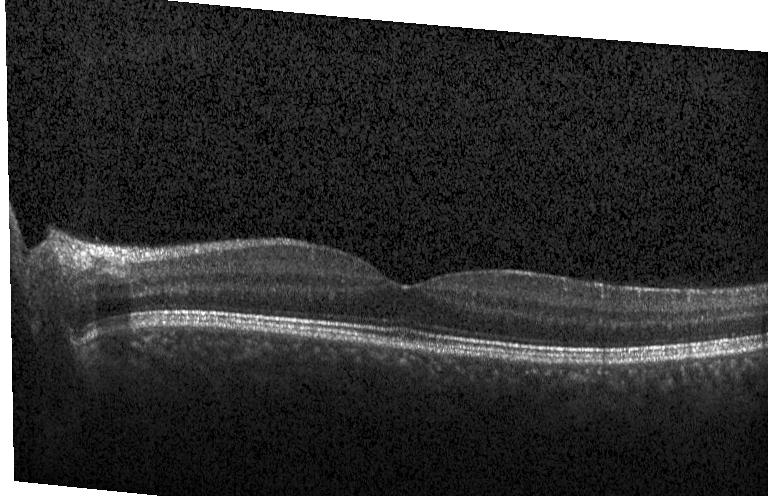 Macular OCT: no evidence of choroidal neovascularization, diabetic macular edema, or drusen.